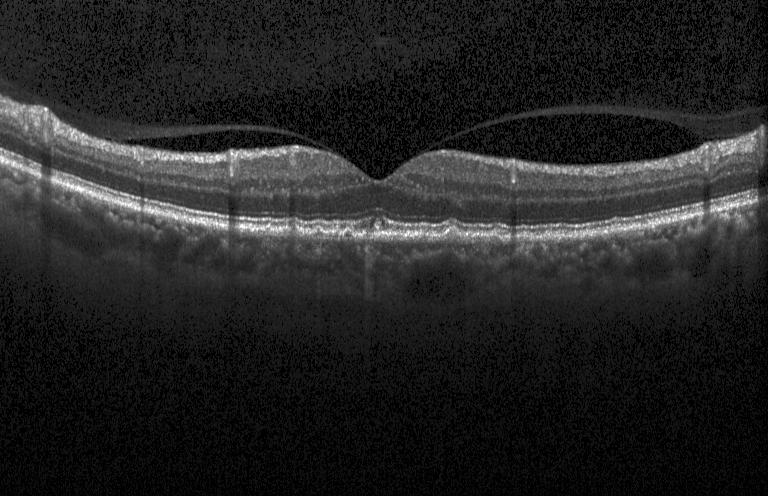

Retinal OCT cross-section, macular scan, Heidelberg Spectralis OCT system, spectral-domain optical coherence tomography — OCT finding: sub-RPE drusenoid deposits.